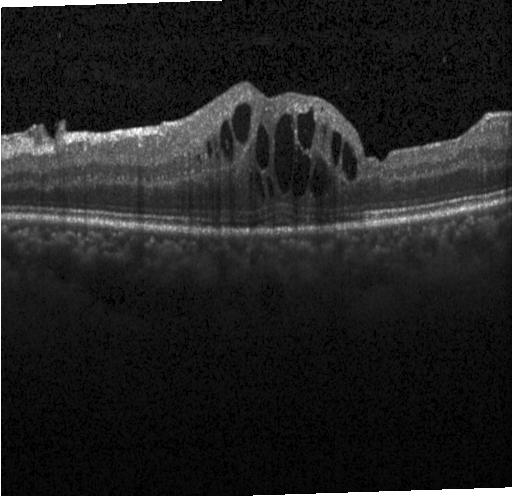 Instrument: Heidelberg Spectralis, spectral-domain optical coherence tomography, retinal OCT B-scan. Assessment: diabetic macular edema.